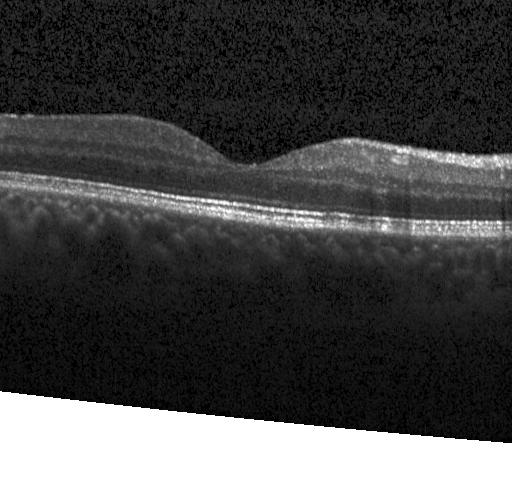
Centered on the fovea · optical coherence tomography B-scan · spectral-domain OCT · Heidelberg Spectralis OCT system — Dx: no choroidal neovascularization, no diabetic macular edema, and no drusen.